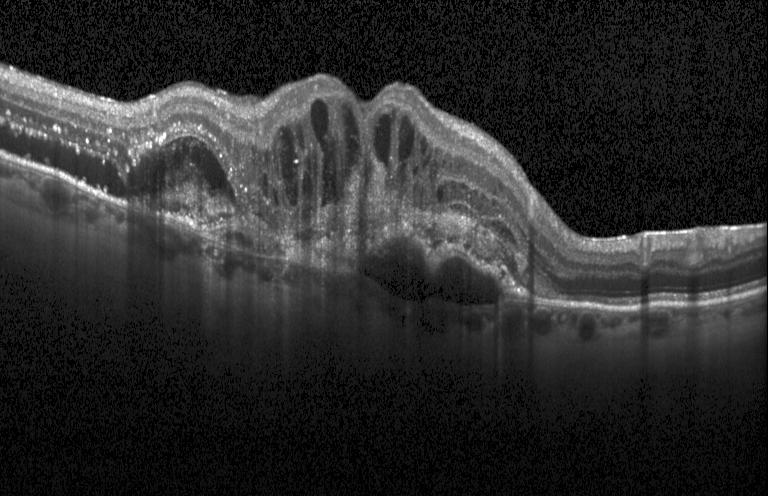 SD-OCT, optical coherence tomography scan, horizontal scan through the fovea — A choroidal neovascular membrane.